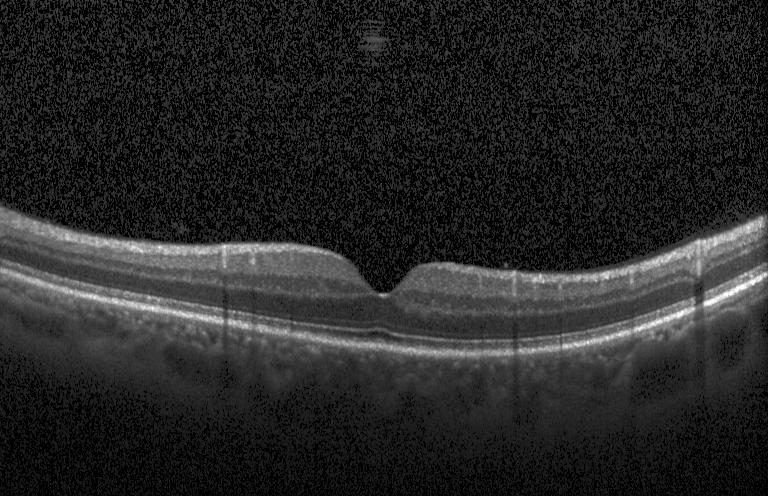
The scan shows neither choroidal neovascularization, diabetic macular edema, nor drusen.